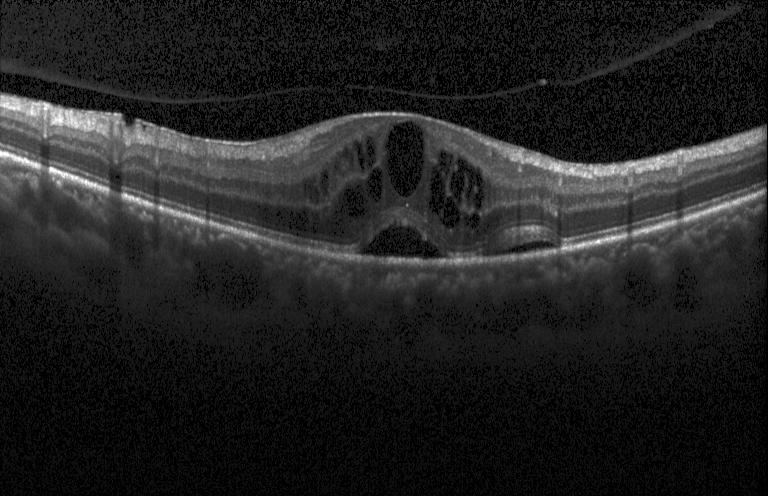 Retinal OCT cross-section; spectral-domain optical coherence tomography; instrument: Heidelberg Spectralis.
Diabetic macular edema (DME).